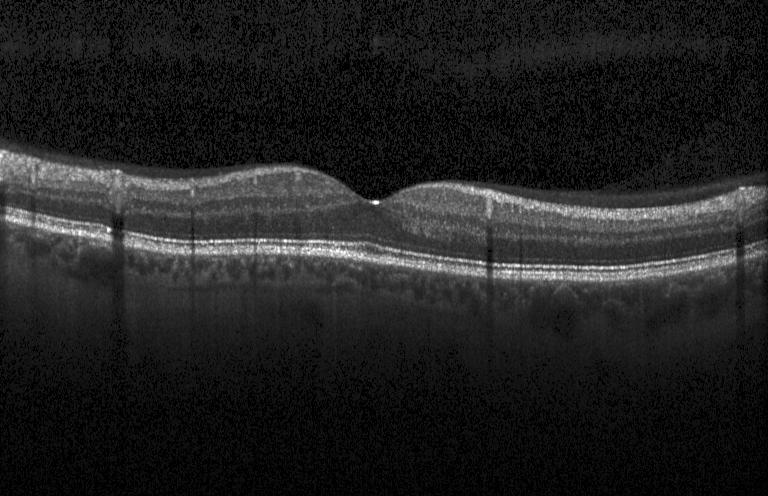
OCT line scan — Dx: no choroidal neovascularization, diabetic macular edema, or drusen.